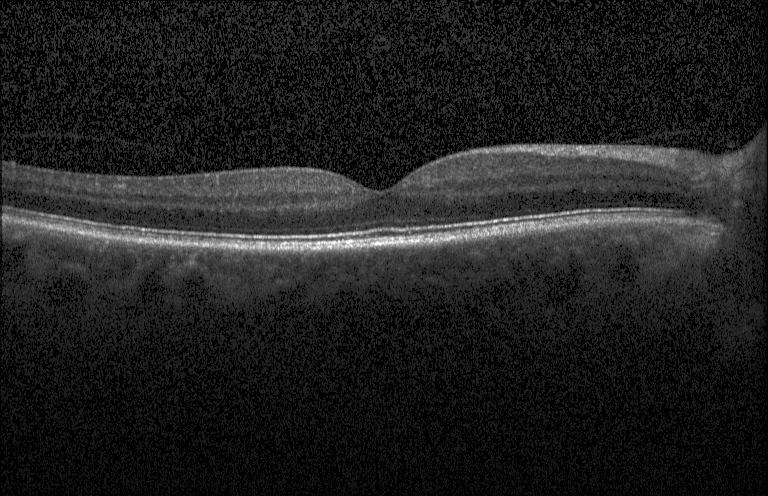
Retinal OCT cross-section showing no evidence of choroidal neovascularization, diabetic macular edema, or drusen.